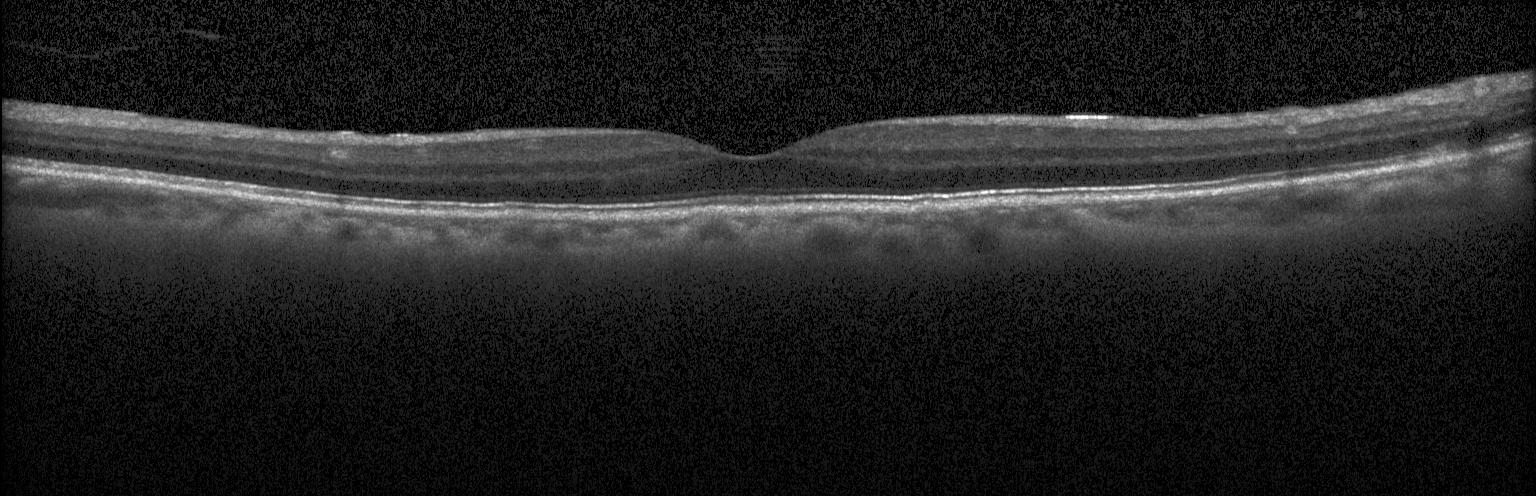

OCT line scan, horizontal scan through the fovea, SD-OCT. Diagnosis: neither choroidal neovascularization, diabetic macular edema, nor drusen.